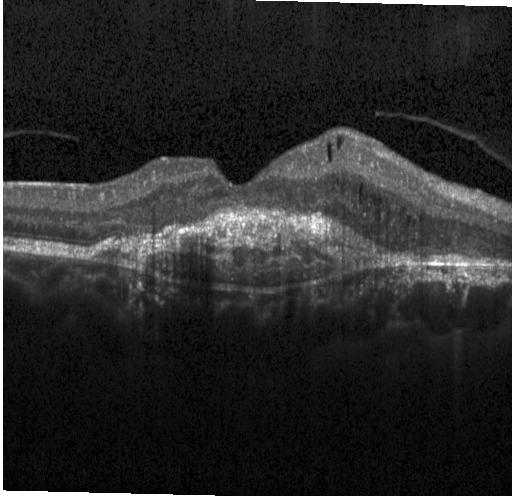 Macular OCT: a choroidal neovascular membrane.